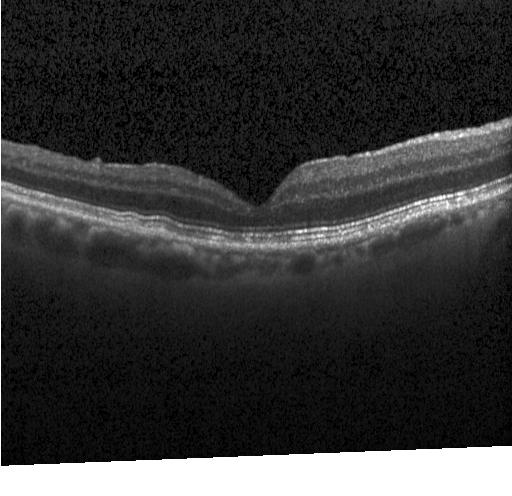 Retinal OCT cross-section, through the macula — This B-scan demonstrates neither choroidal neovascularization, diabetic macular edema, nor drusen.